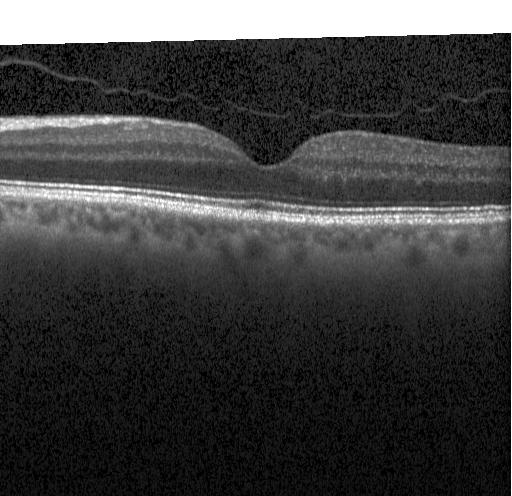 OCT B-scan.
Finding: no evidence of choroidal neovascularization, diabetic macular edema, or drusen.